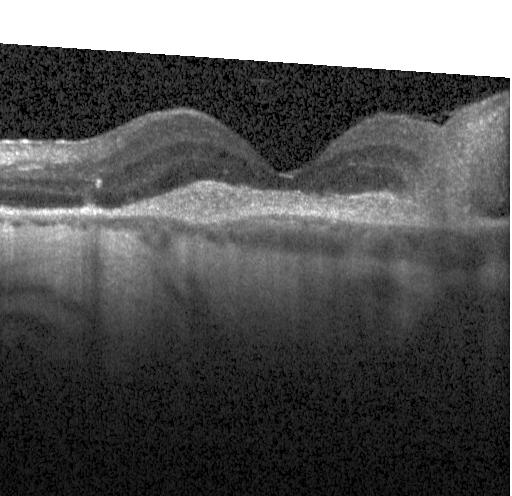

OCT B-scan showing choroidal neovascularization (CNV).